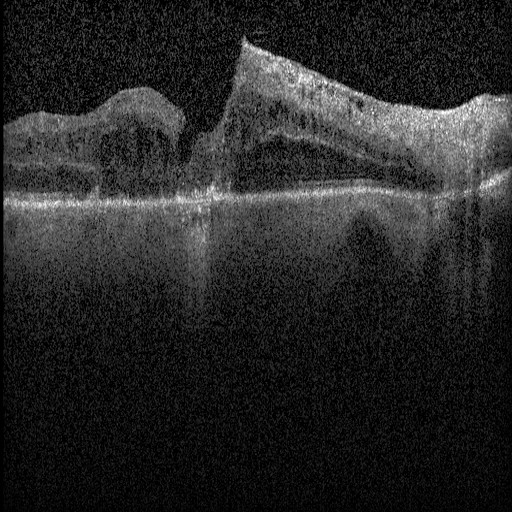

Optical coherence tomography scan — Diagnosis: diabetic macular edema (DME).